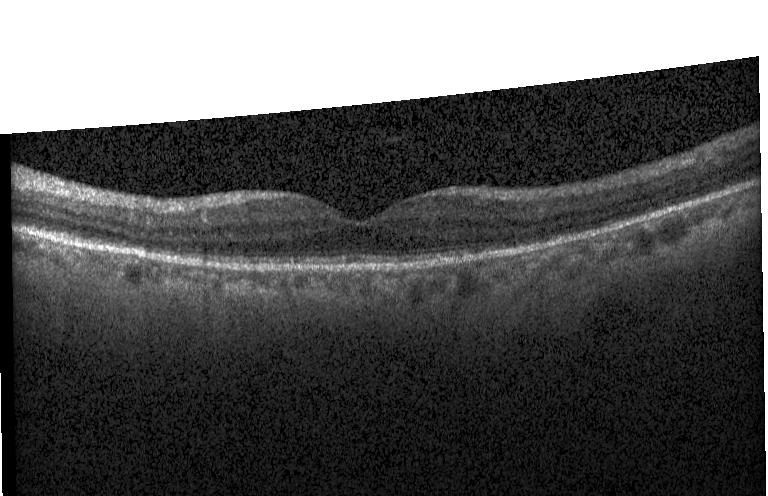

Spectral-domain OCT B-scan: no CNV, DME, or drusen.